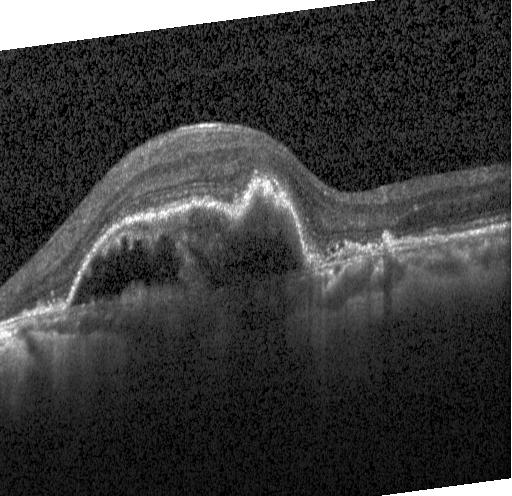

Spectral-domain OCT; through the macula; Heidelberg Spectralis; optical coherence tomography scan — Macular OCT: a choroidal neovascular membrane.